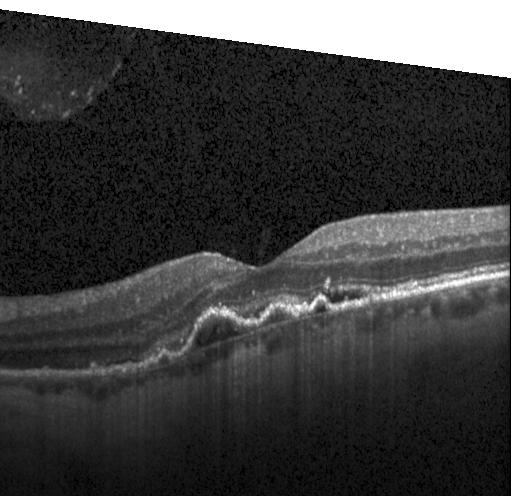

Dx: choroidal neovascularization (CNV).